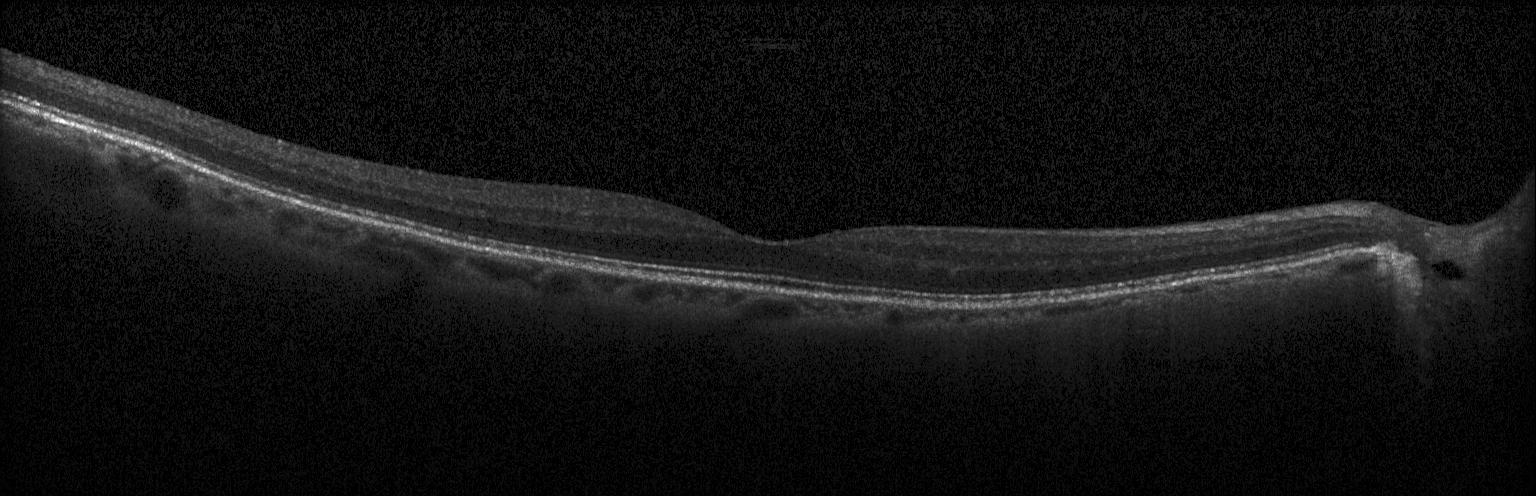

Assessment: no evidence of choroidal neovascularization, diabetic macular edema, or drusen.